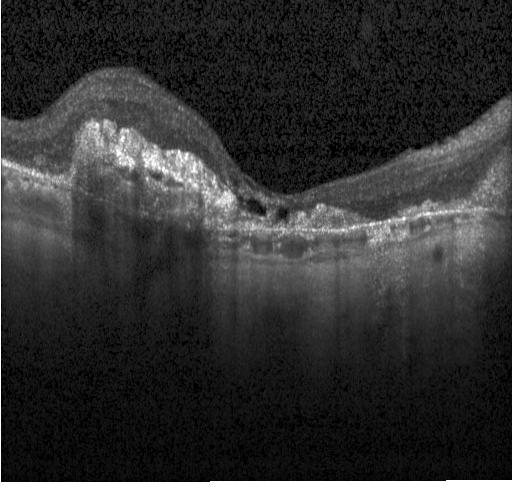

Heidelberg Spectralis. Optical coherence tomography B-scan — Diagnosis: a choroidal neovascular membrane.